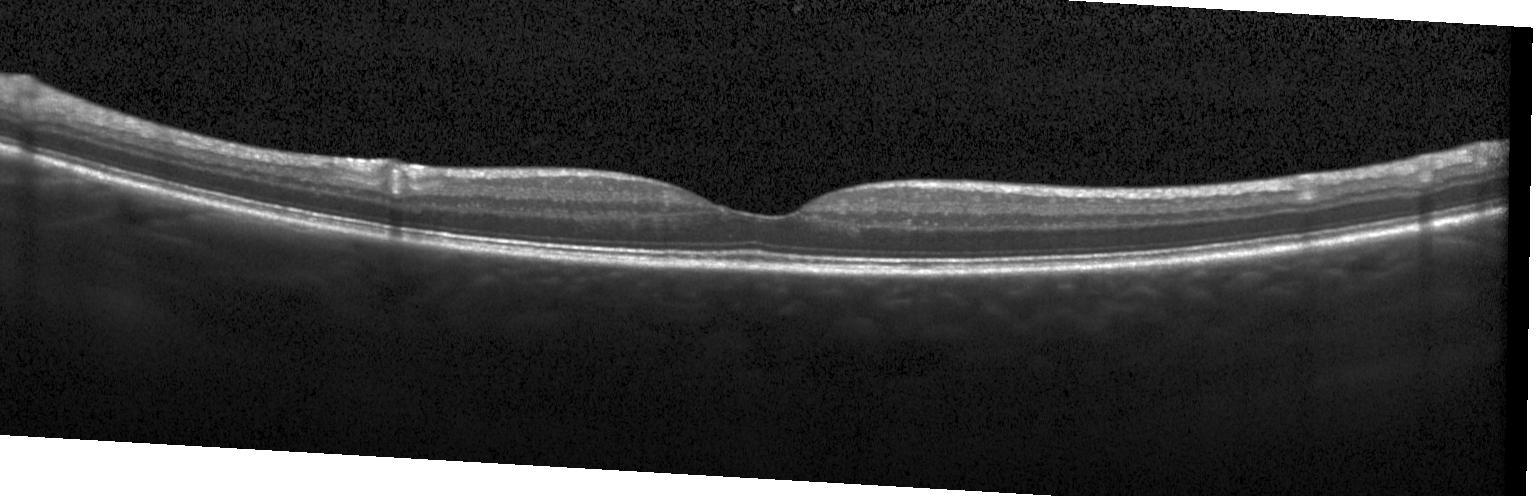

Retinal OCT B-scan. Heidelberg Spectralis OCT system
Diagnosis: no CNV, no DME, and no drusen.